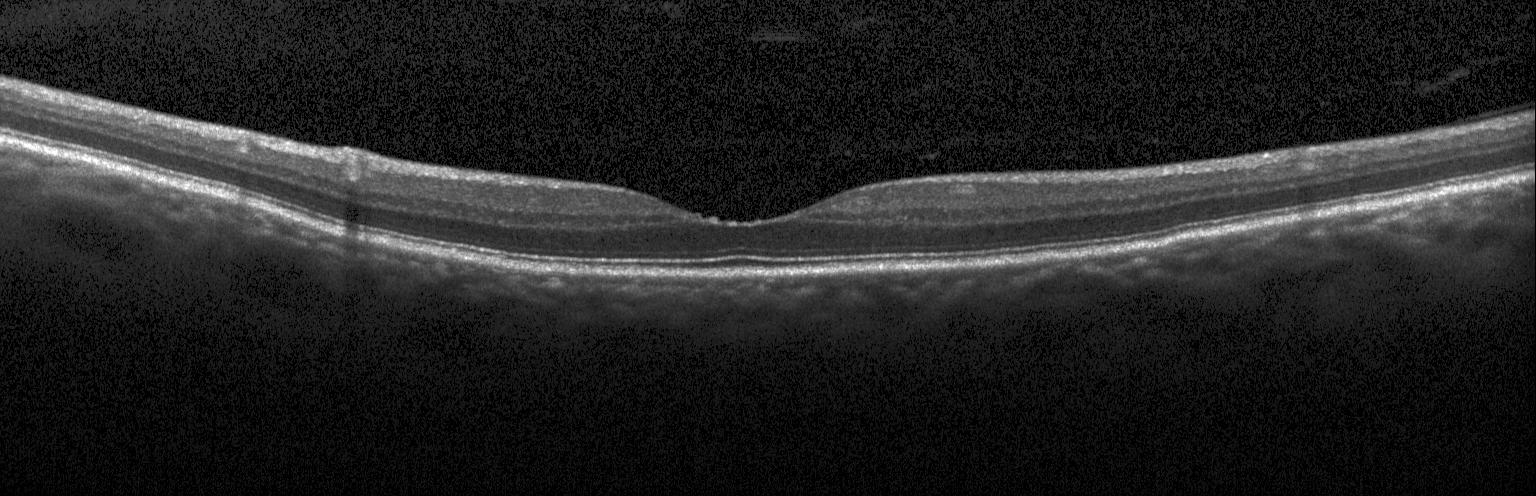

Spectral-domain optical coherence tomography; Heidelberg Spectralis; optical coherence tomography B-scan; horizontal scan through the fovea. Finding: no evidence of CNV, DME, or drusen.